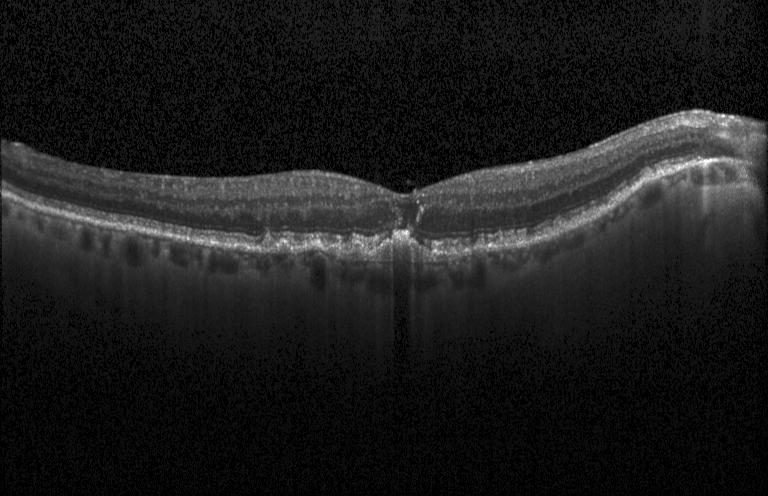

Retinal OCT B-scan — Finding: sub-RPE drusenoid deposits.